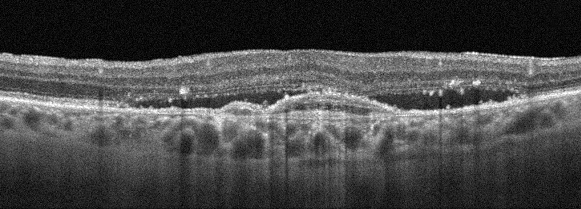
Left eye; OCT line scan — Finding: age-related macular degeneration (AMD).